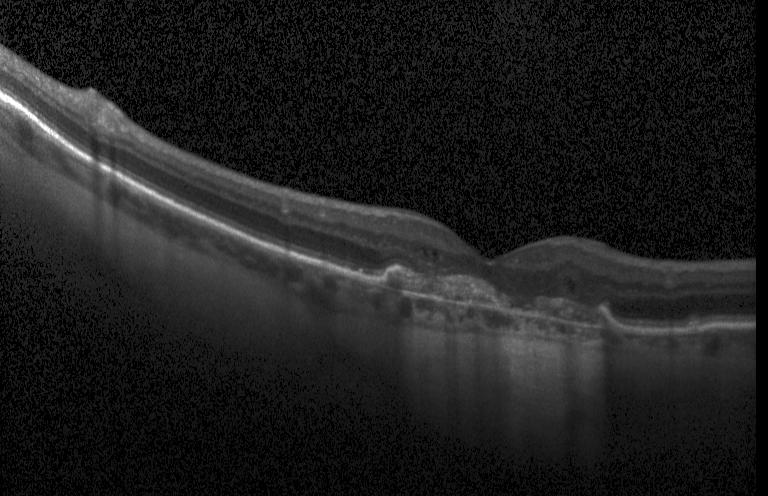 Impression: a choroidal neovascular membrane.